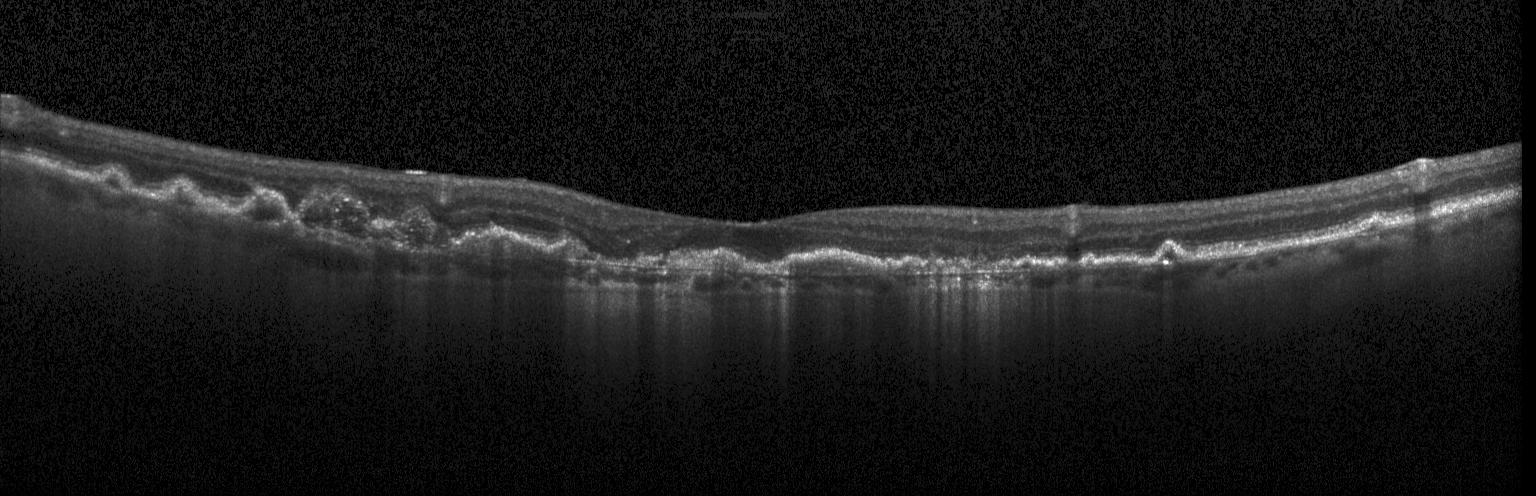
Acquired on a Heidelberg Spectralis; OCT line scan — OCT finding: a choroidal neovascular membrane.